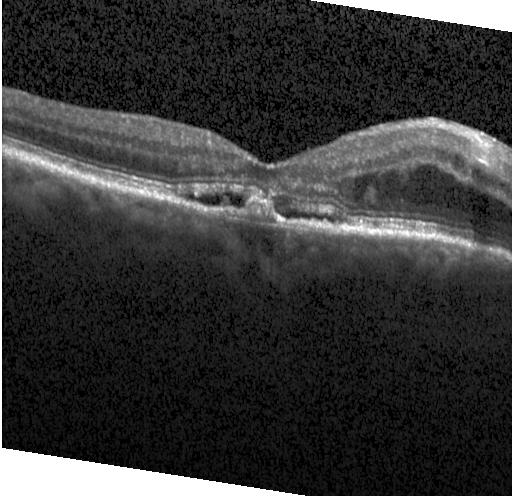
Macular scan. Spectral-domain optical coherence tomography. OCT B-scan.
Macular OCT: a choroidal neovascular membrane.